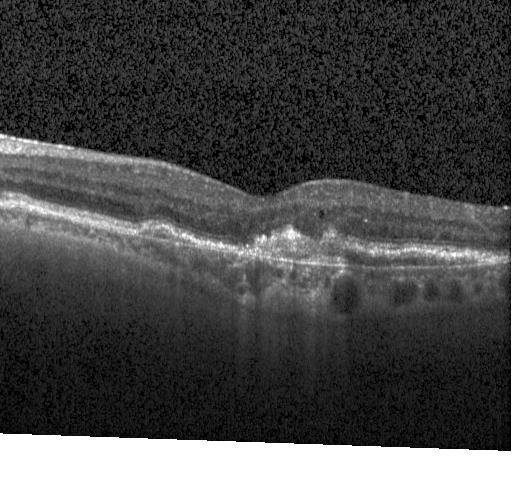 Acquired on a Heidelberg Spectralis. SD-OCT. Optical coherence tomography B-scan. Through the macula. Finding: CNV.